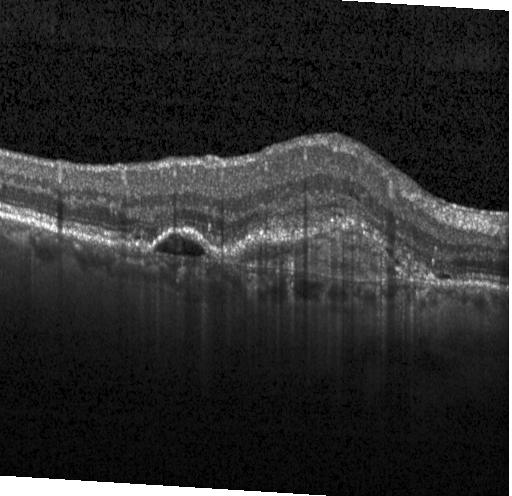 Optical coherence tomography scan
Finding: a choroidal neovascular membrane.